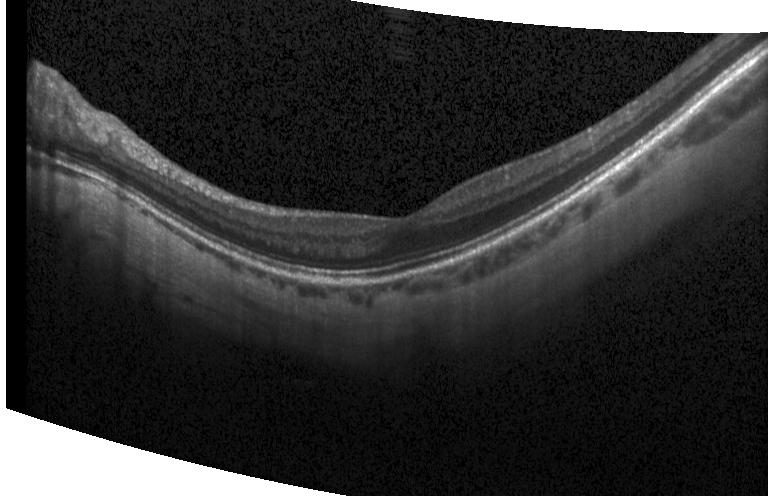 This B-scan demonstrates no choroidal neovascularization, diabetic macular edema, or drusen.